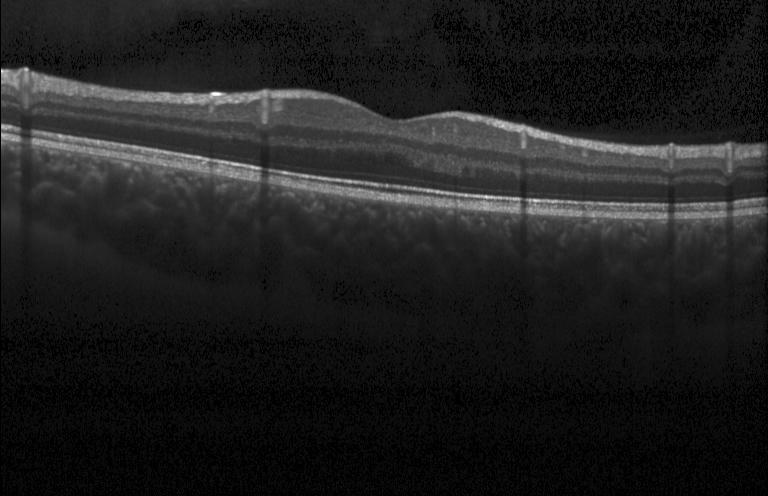
Instrument: Heidelberg Spectralis. Retinal OCT B-scan
Diagnosis: neither CNV, DME, nor drusen.